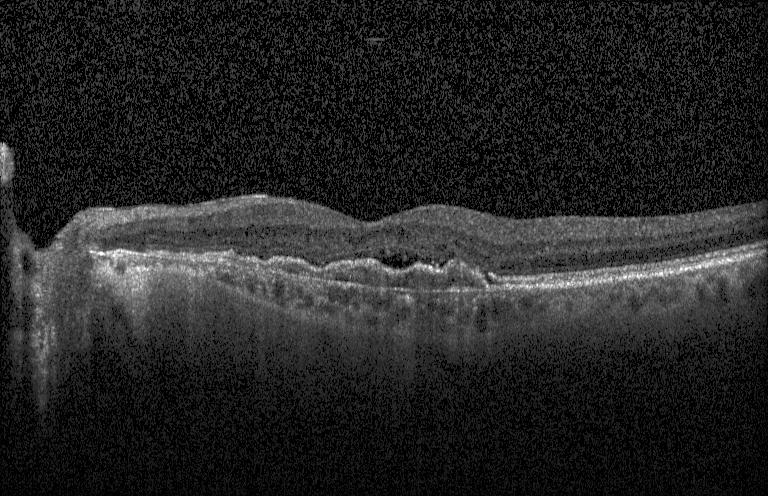

Optical coherence tomography B-scan; through the macula.
Impression: choroidal neovascularization (CNV).